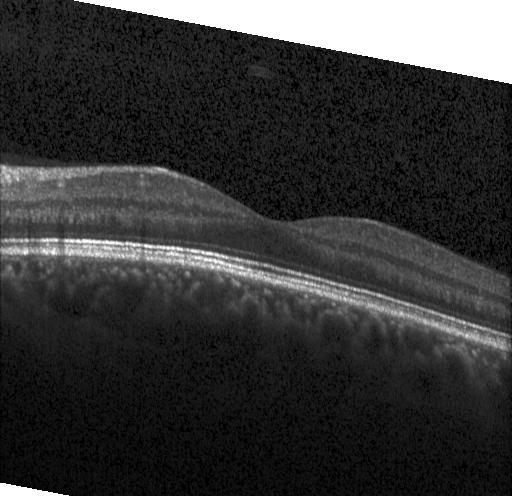

Optical coherence tomography scan.
The scan shows no choroidal neovascularization, diabetic macular edema, or drusen.